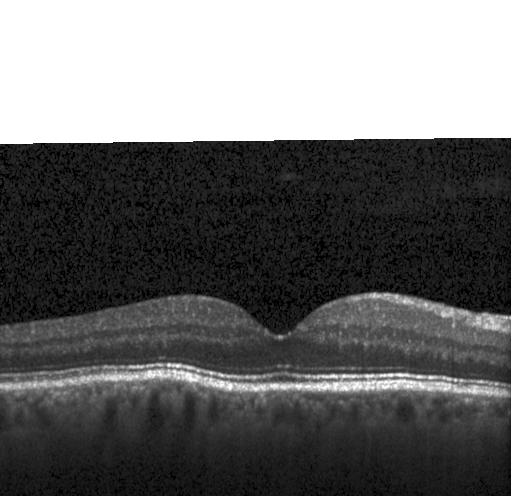 OCT B-scan
Diagnosis: no evidence of choroidal neovascularization, diabetic macular edema, or drusen.